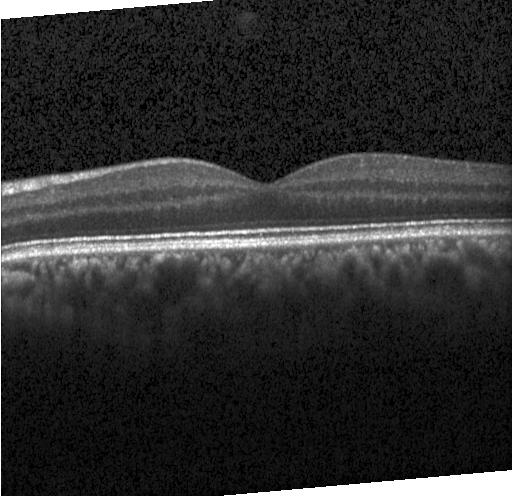

OCT scan showing neither choroidal neovascularization, diabetic macular edema, nor drusen.